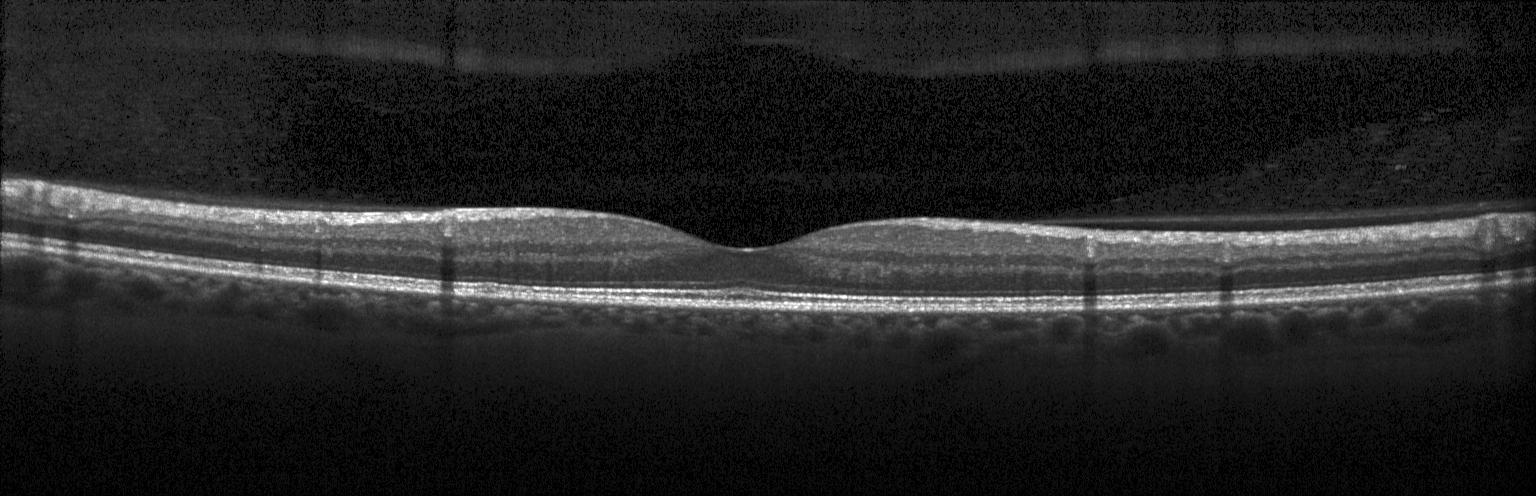

Dx: no evidence of choroidal neovascularization, diabetic macular edema, or drusen.